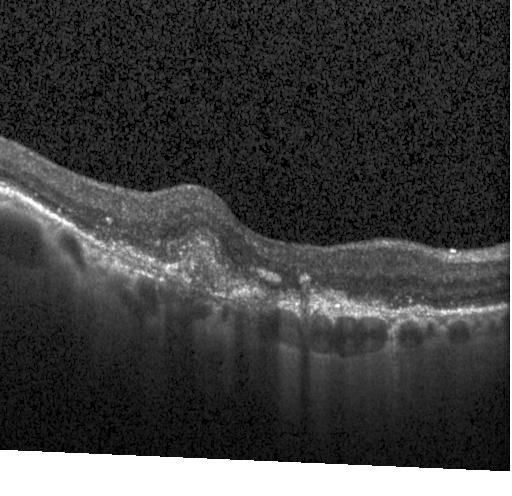

Spectral-domain optical coherence tomography, OCT B-scan. Impression: a choroidal neovascular membrane.